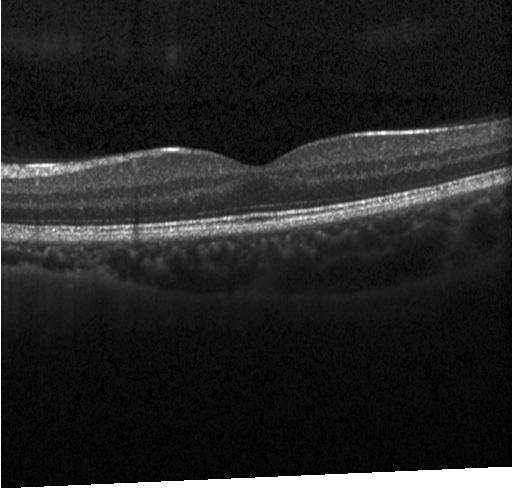
Assessment: no CNV, DME, or drusen.